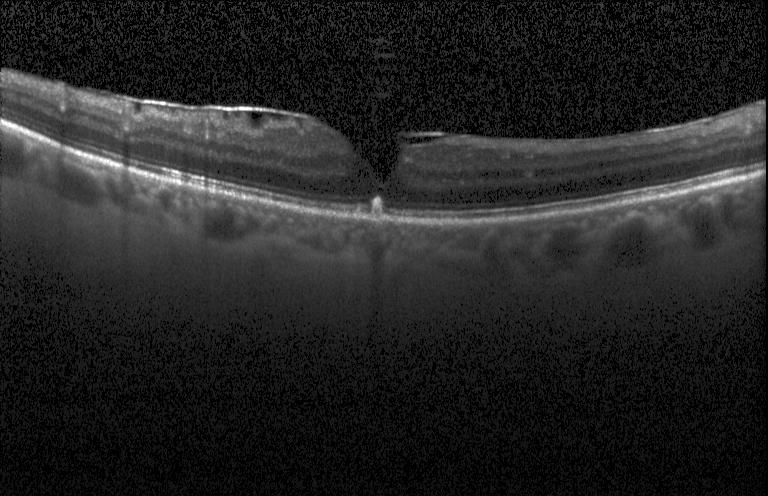 Retinal OCT cross-section showing drusen.